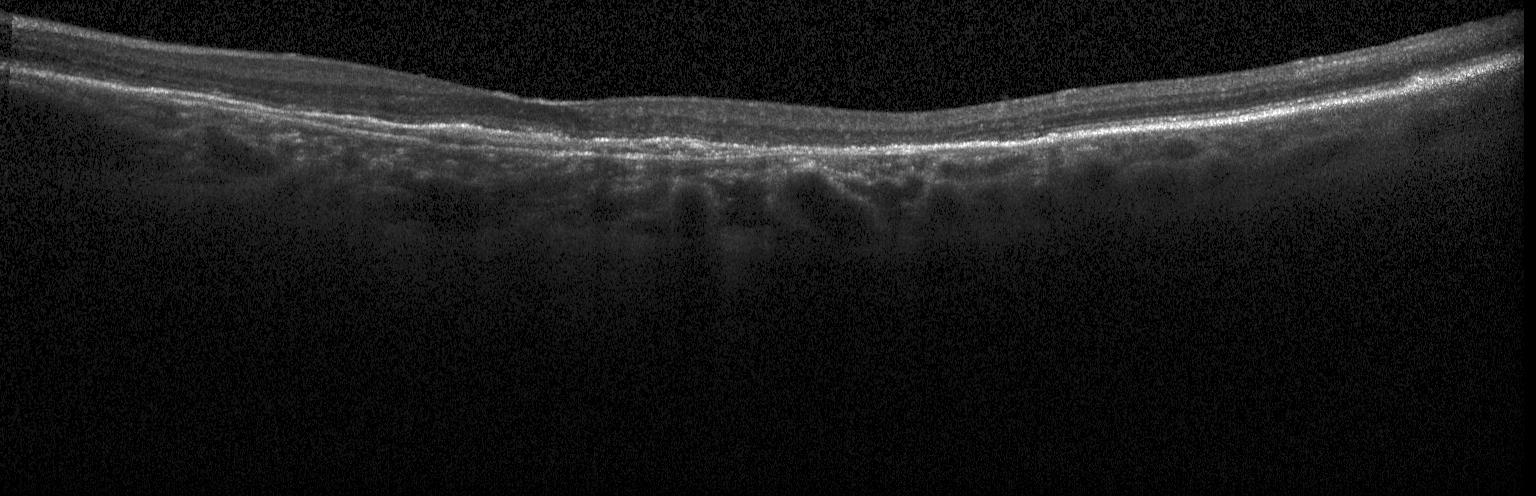
Optical coherence tomography B-scan · through the macula · acquired on a Heidelberg Spectralis · spectral-domain OCT.
Diagnosis: choroidal neovascularization.